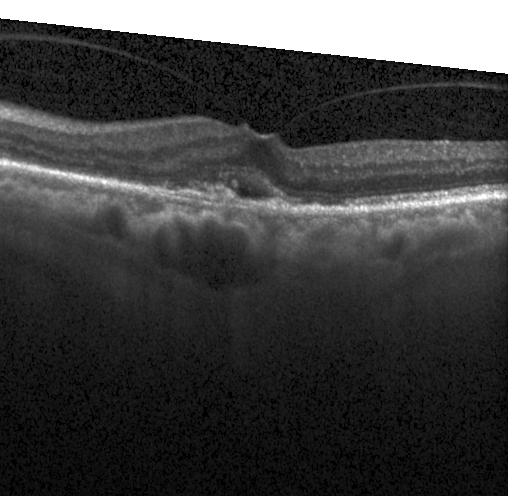
Finding: a choroidal neovascular membrane.